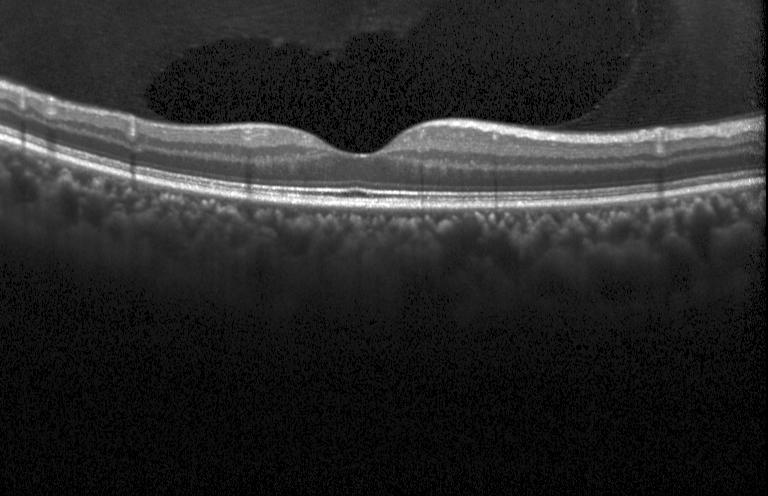
Instrument: Heidelberg Spectralis. Macular scan. Retinal OCT B-scan. Spectral-domain OCT — OCT finding: neither choroidal neovascularization, diabetic macular edema, nor drusen.